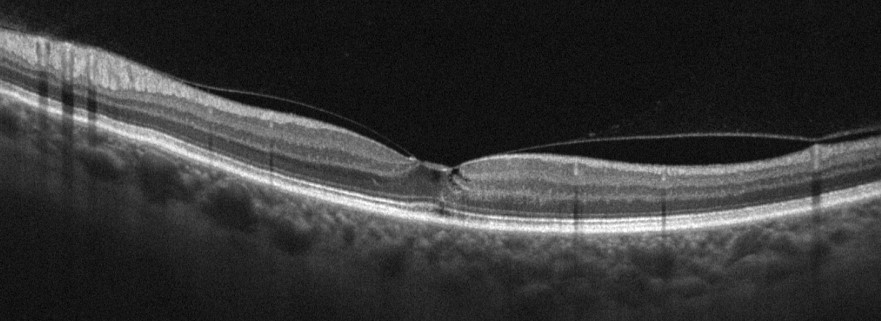

Macular scan; OCT B-scan.
Diagnosis: vitreomacular interface disease (VID).